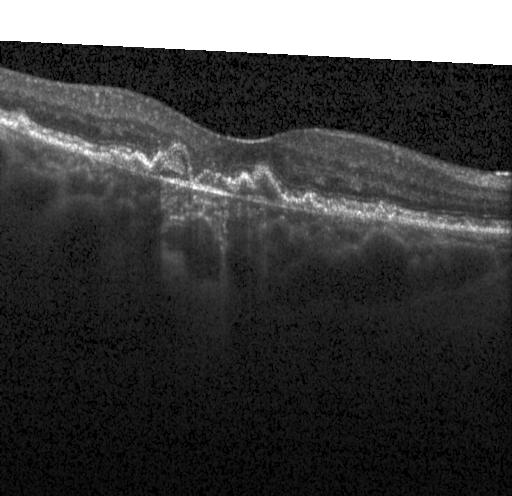 Macular OCT: a choroidal neovascular membrane.